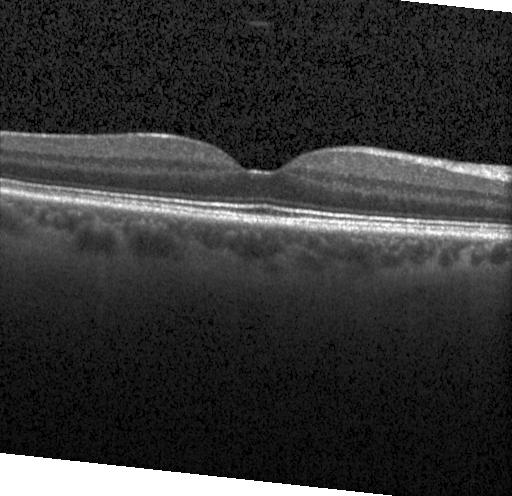 Impression: no choroidal neovascularization, no diabetic macular edema, and no drusen.